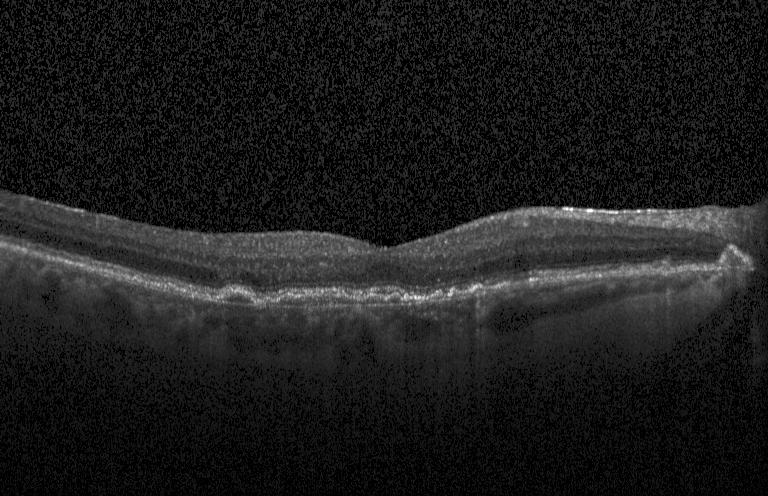 Diagnosis: choroidal neovascularization (CNV).